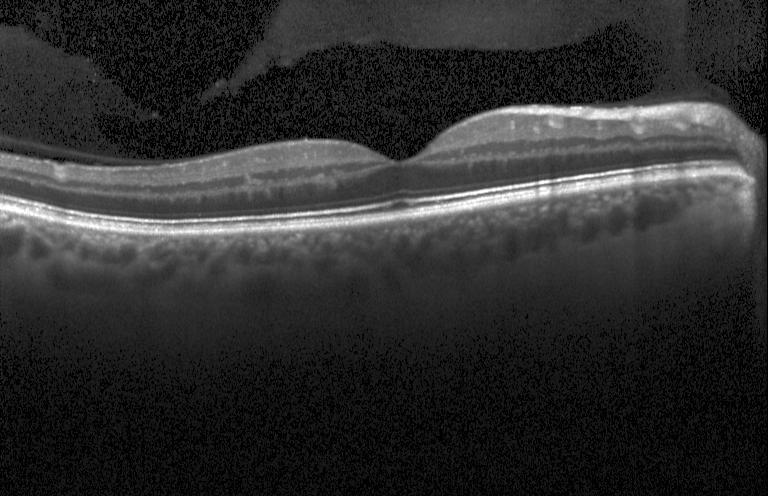

Horizontal scan through the fovea, optical coherence tomography scan
The scan shows neither CNV, DME, nor drusen.